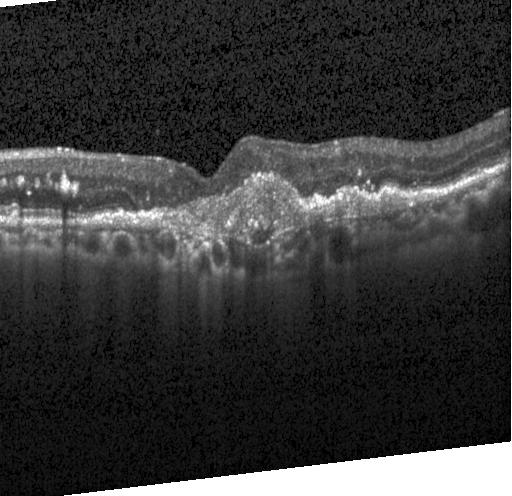
OCT line scan.
Dx: choroidal neovascularization.